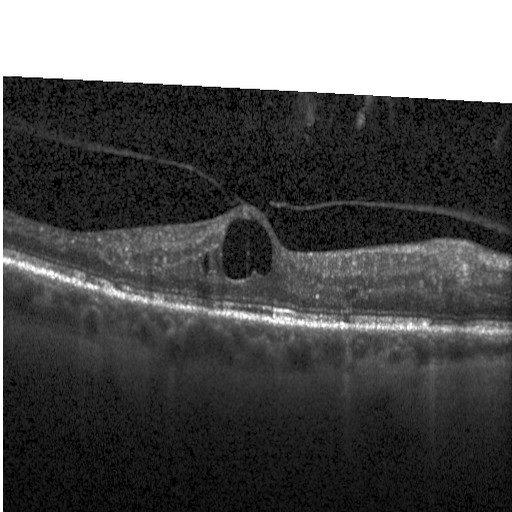
Retinal OCT cross-section; instrument: Heidelberg Spectralis; horizontal scan through the fovea
Impression: DME.